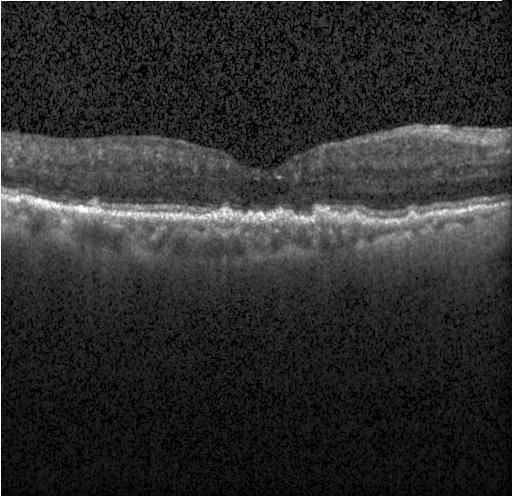

OCT scan showing multiple drusen.